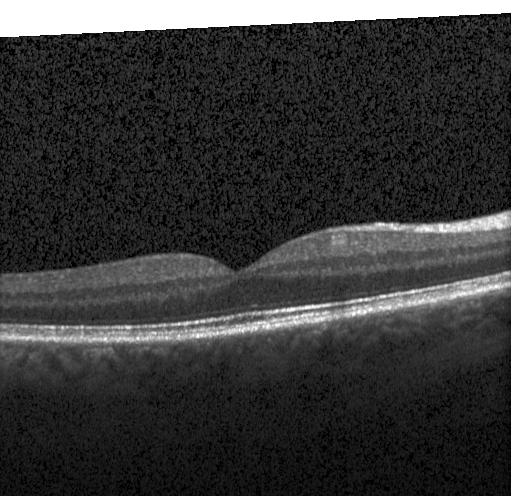
Macular scan; optical coherence tomography B-scan; acquired on a Heidelberg Spectralis; spectral-domain optical coherence tomography.
No evidence of choroidal neovascularization, diabetic macular edema, or drusen.